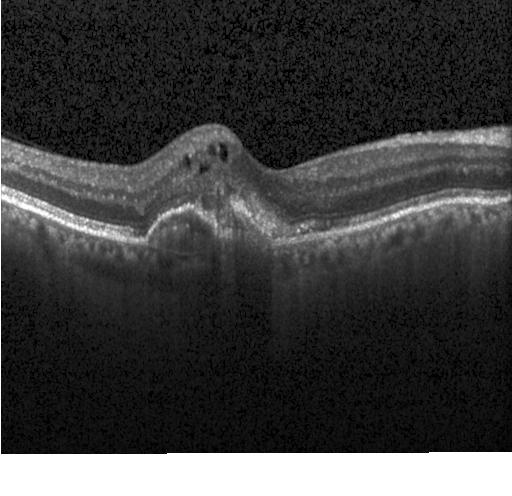
Horizontal scan through the fovea · retinal OCT cross-section · SD-OCT. Impression: CNV.